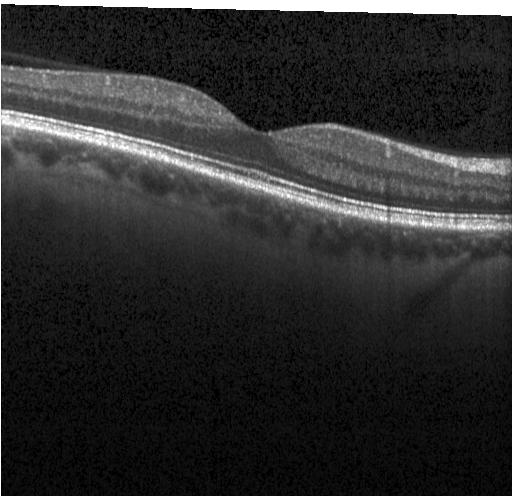

SD-OCT; optical coherence tomography B-scan; horizontal scan through the fovea
The scan shows no choroidal neovascularization, no diabetic macular edema, and no drusen.